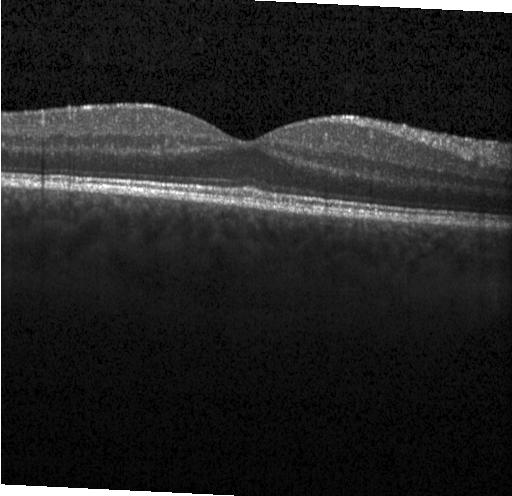

Heidelberg Spectralis. Optical coherence tomography scan
OCT finding: no evidence of choroidal neovascularization, diabetic macular edema, or drusen.